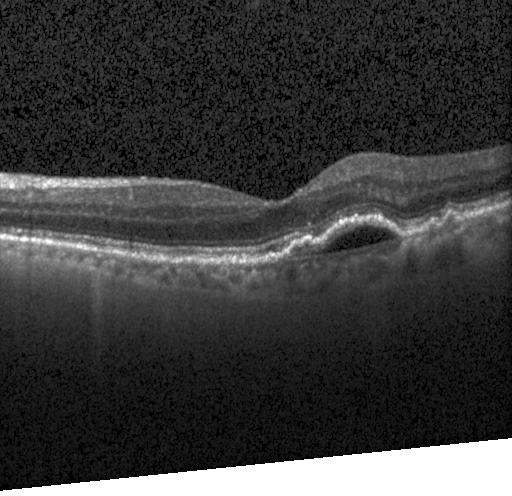
Retinal OCT B-scan, through the macula, spectral-domain OCT.
OCT finding: CNV.